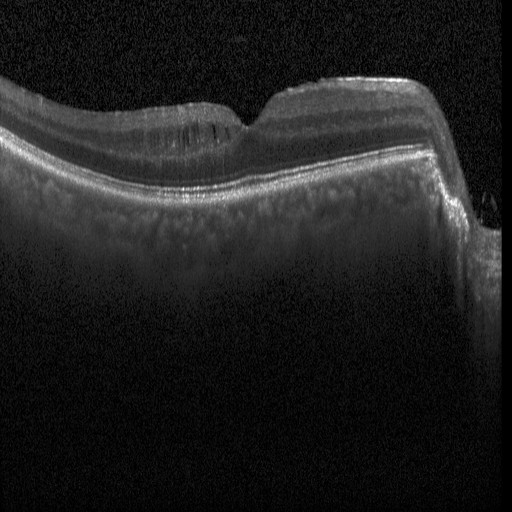

Impression: DME.